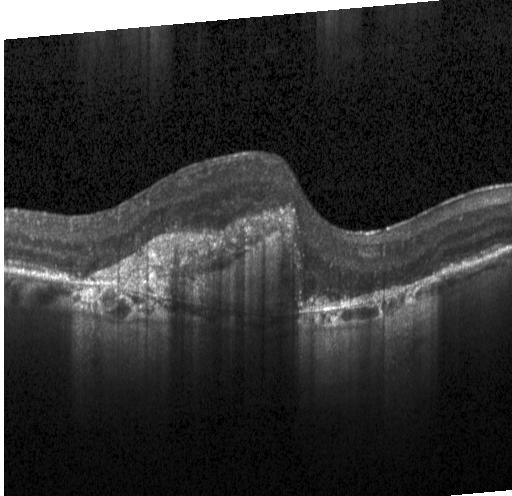
Retinal OCT B-scan · instrument: Heidelberg Spectralis · fovea-centered · SD-OCT — Diagnosis: a choroidal neovascular membrane.